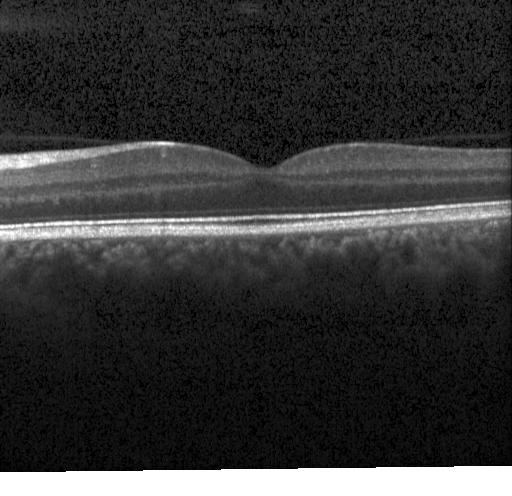

Retinal OCT cross-section
Finding: no choroidal neovascularization, no diabetic macular edema, and no drusen.